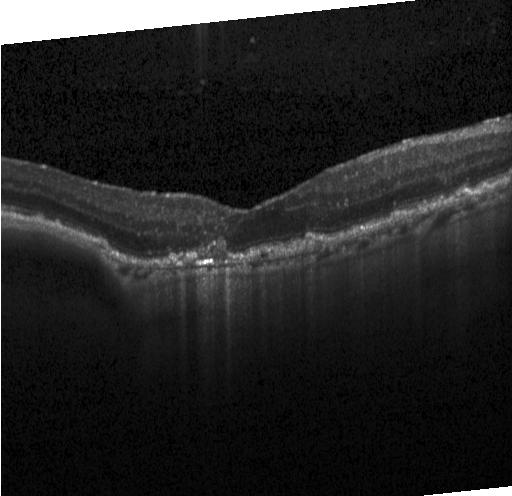

Diagnosis: CNV.